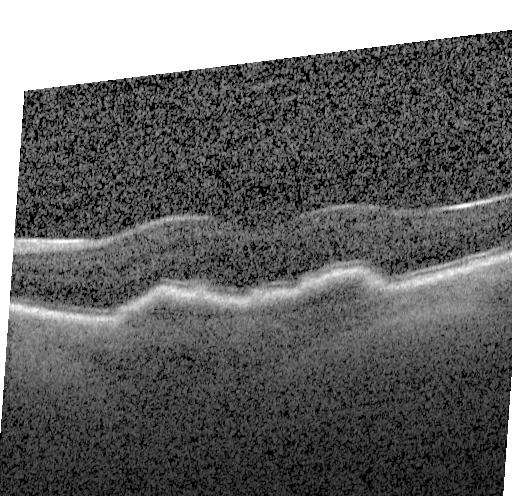

Impression: a choroidal neovascular membrane.